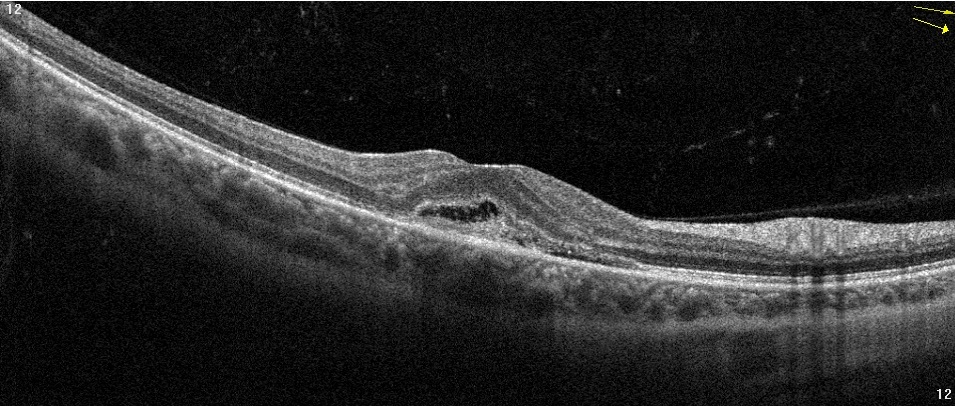
Acquired on an Optovue Avanti RTVue XR. Retinal OCT B-scan. Fovea-centered — Diagnosis: AMD.